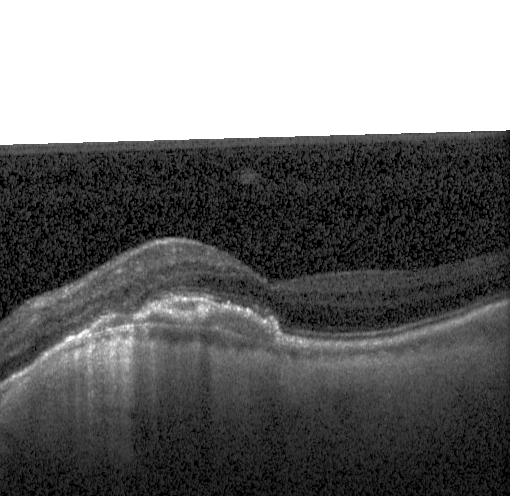
Instrument: Heidelberg Spectralis; optical coherence tomography B-scan; macular scan; SD-OCT.
Finding: a choroidal neovascular membrane.